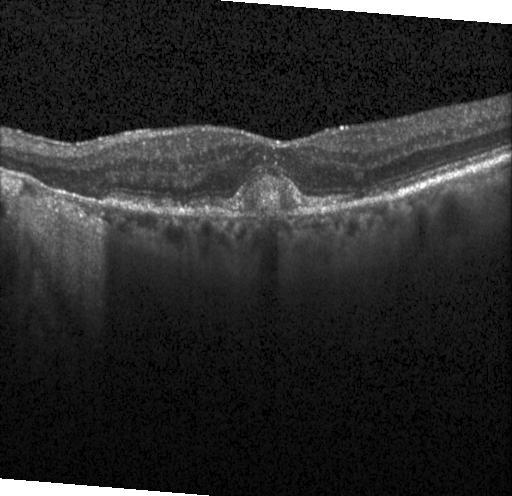

Diagnosis: choroidal neovascularization (CNV).